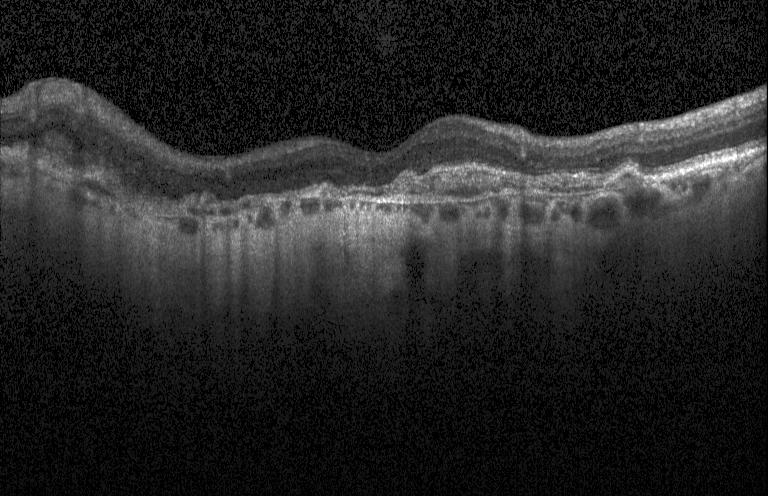 Retinal OCT cross-section — Finding: CNV.